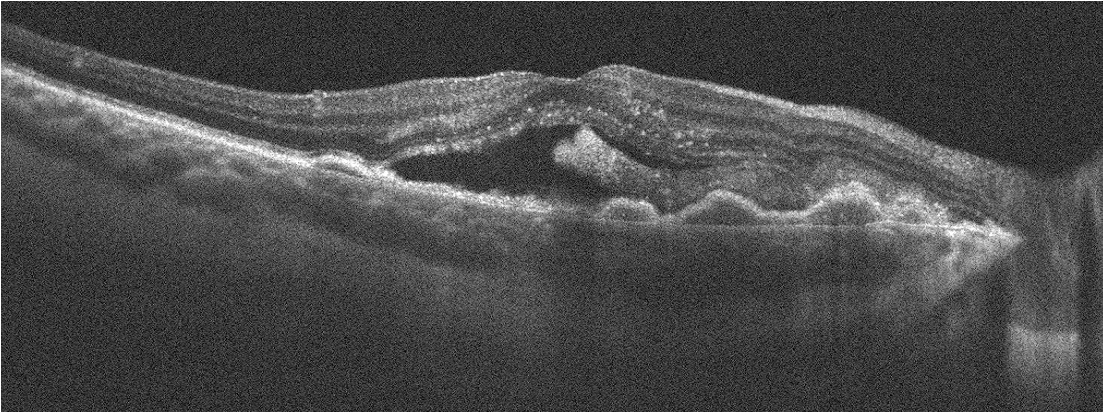
Retinal OCT cross-section; instrument: Optovue Avanti RTVue XR — Finding: age-related macular degeneration.